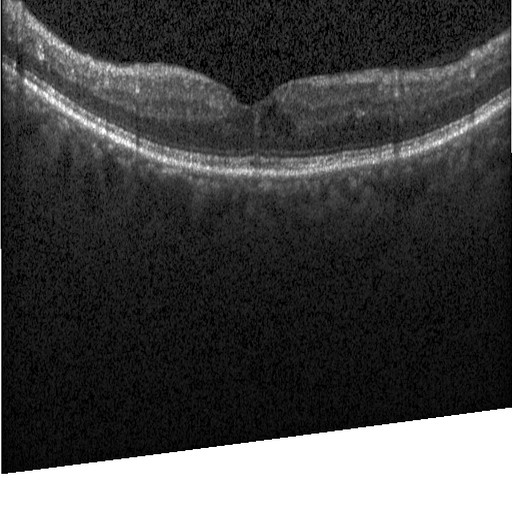 OCT B-scan; instrument: Heidelberg Spectralis; centered on the fovea.
The scan shows diabetic macular edema (DME).